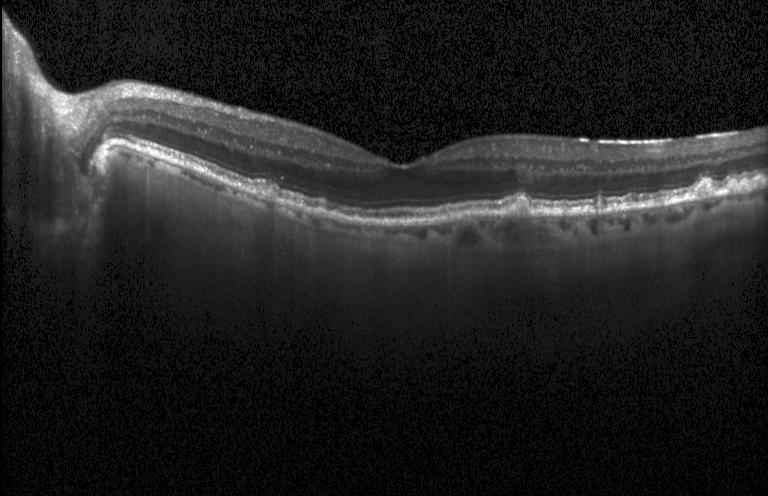

Diagnosis: drusen.